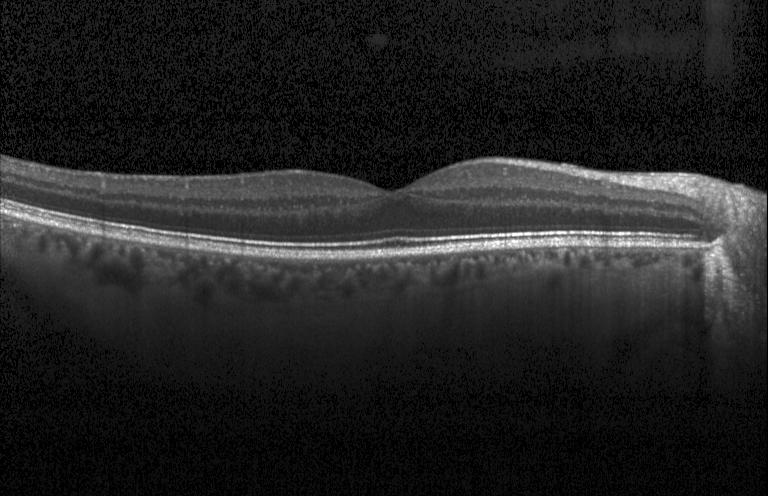 SD-OCT. Fovea-centered. OCT B-scan. The scan shows no evidence of choroidal neovascularization, diabetic macular edema, or drusen.